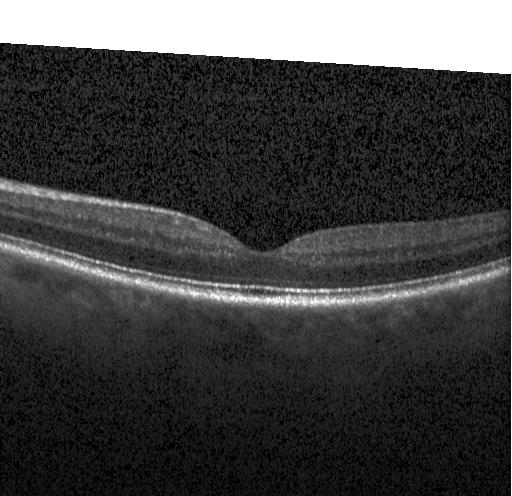 Retinal OCT cross-section, Heidelberg Spectralis
This B-scan demonstrates no choroidal neovascularization, diabetic macular edema, or drusen.